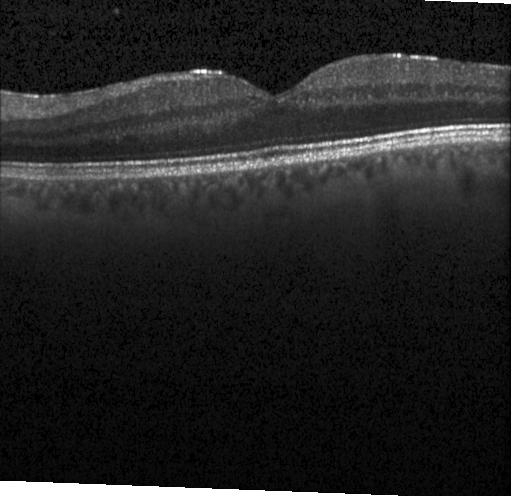
Diagnosis: no choroidal neovascularization, diabetic macular edema, or drusen.